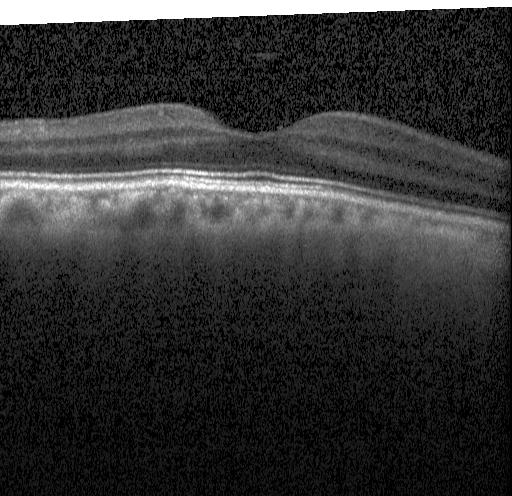

Spectral-domain OCT B-scan: neither CNV, DME, nor drusen.